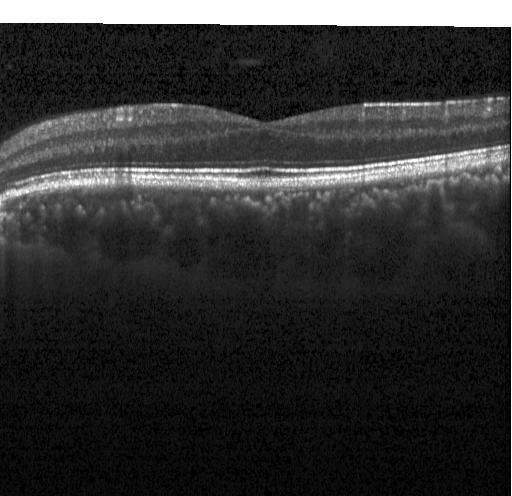
Retinal OCT cross-section. Instrument: Heidelberg Spectralis. Diagnosis: no CNV, no DME, and no drusen.